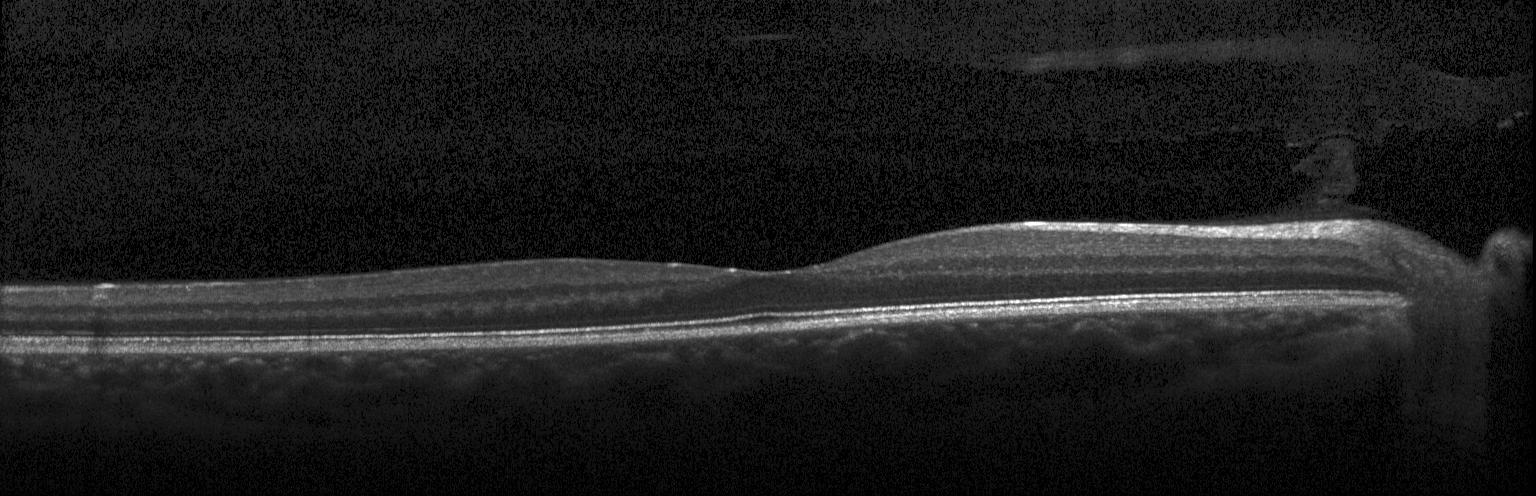 OCT line scan. Impression: neither CNV, DME, nor drusen.